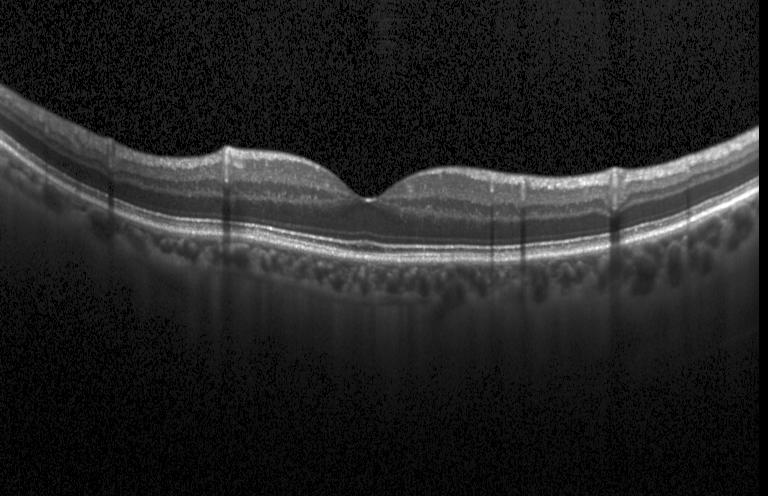
The scan shows neither choroidal neovascularization, diabetic macular edema, nor drusen.